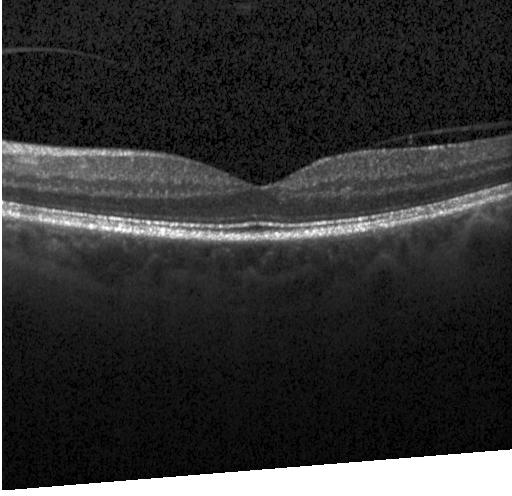 OCT B-scan · SD-OCT · acquired on a Heidelberg Spectralis. Diagnosis: no evidence of CNV, DME, or drusen.